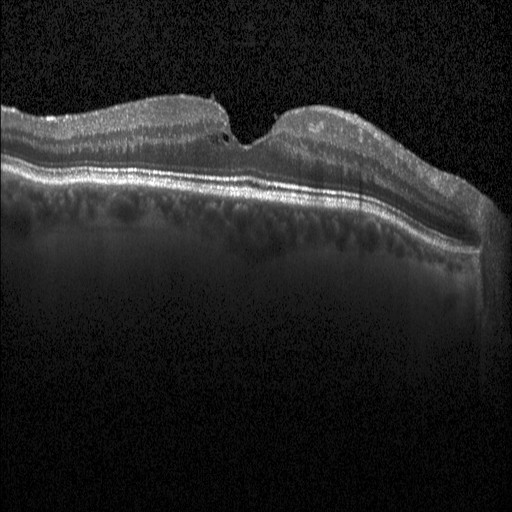 Instrument: Heidelberg Spectralis · OCT B-scan · centered on the fovea · SD-OCT.
Diagnosis: diabetic macular edema.